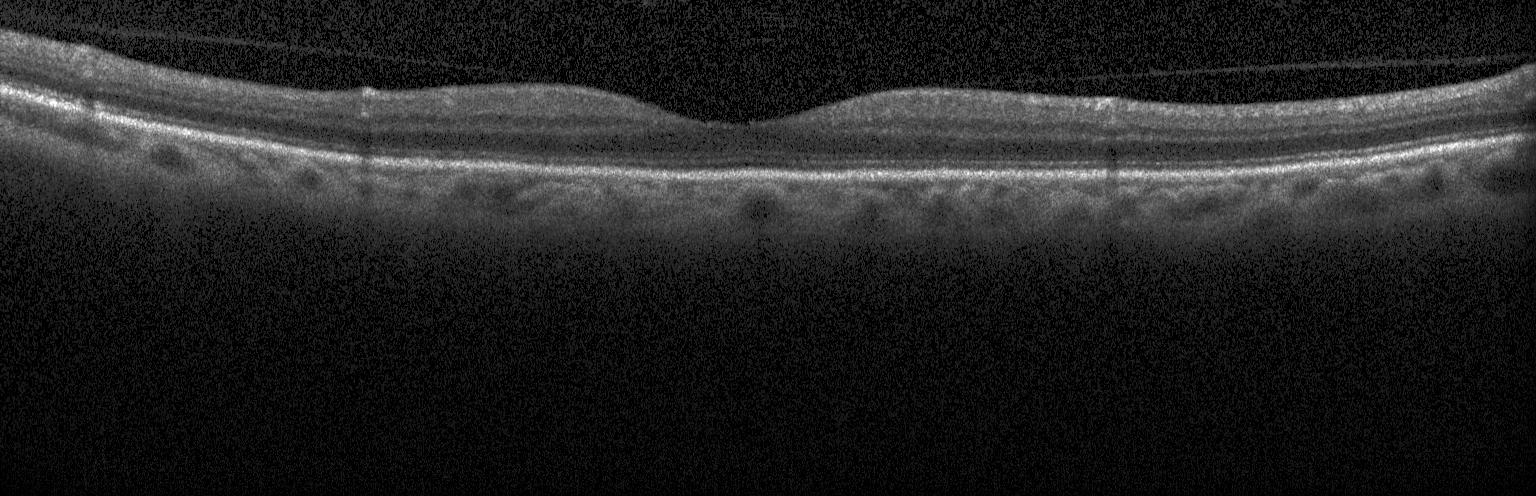 Impression: no evidence of choroidal neovascularization, diabetic macular edema, or drusen.